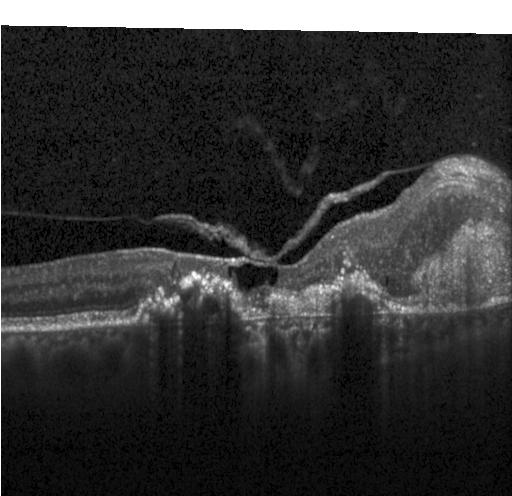

Assessment: choroidal neovascularization (CNV).